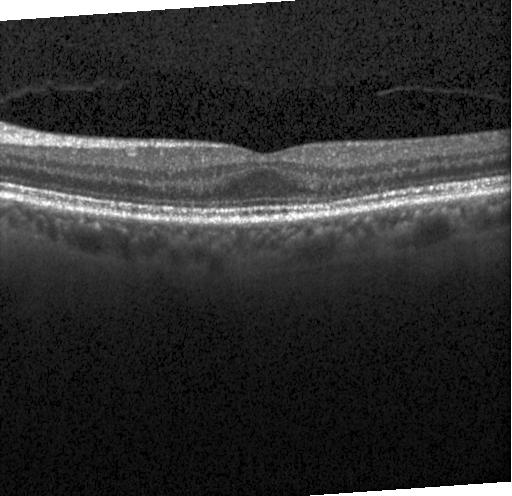 OCT B-scan
Neither choroidal neovascularization, diabetic macular edema, nor drusen.